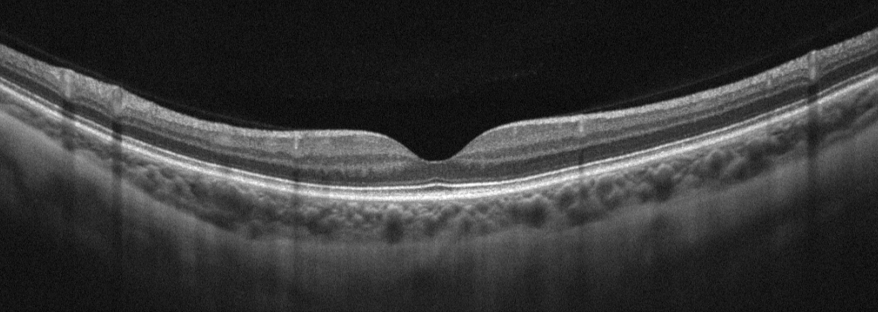

Spectral-domain OCT B-scan: absence of AMD, DME, ERM, RAO, RVO, and vitreomacular interface disease.